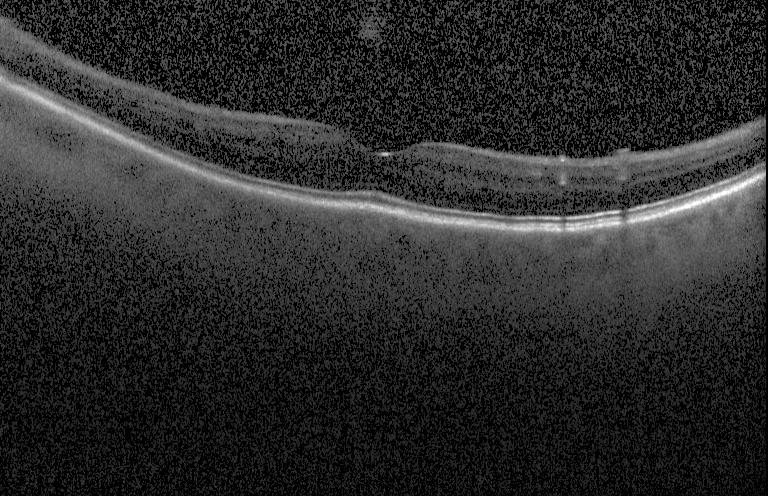 Spectral-domain optical coherence tomography. Retinal OCT B-scan
Impression: neither choroidal neovascularization, diabetic macular edema, nor drusen.